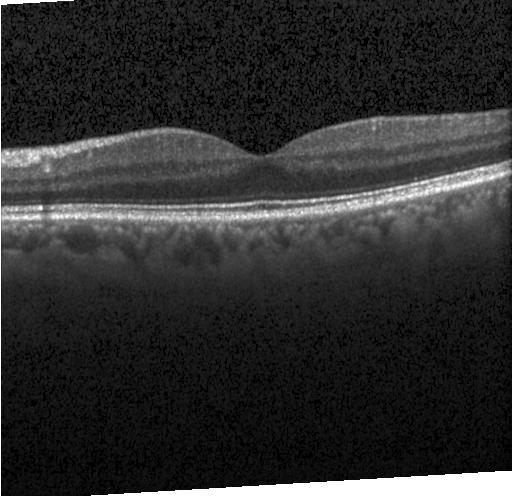 Diagnosis: neither choroidal neovascularization, diabetic macular edema, nor drusen.